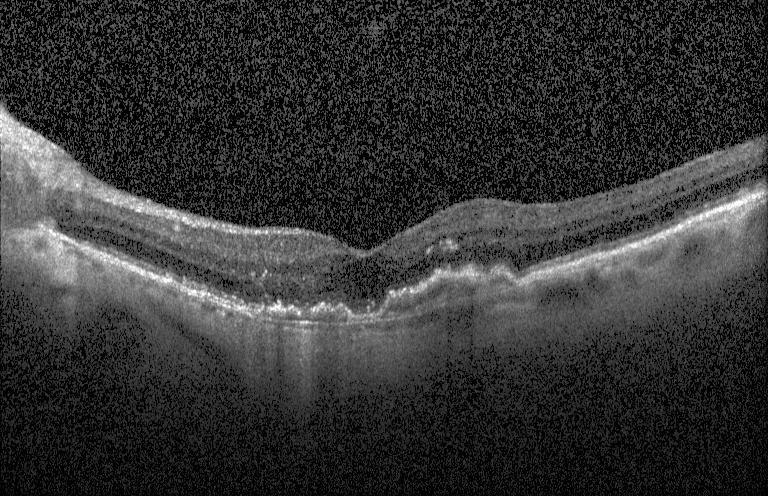

A choroidal neovascular membrane.